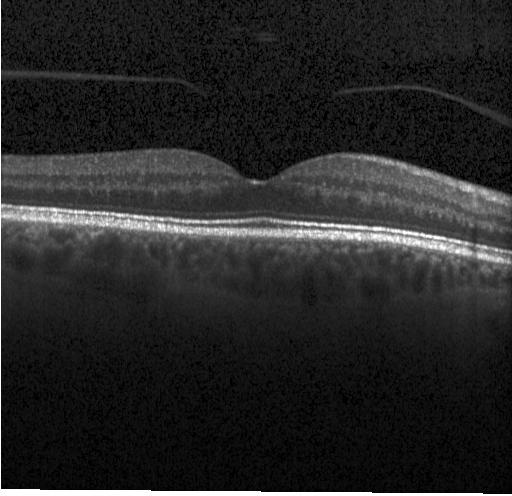
OCT B-scan showing no evidence of choroidal neovascularization, diabetic macular edema, or drusen.